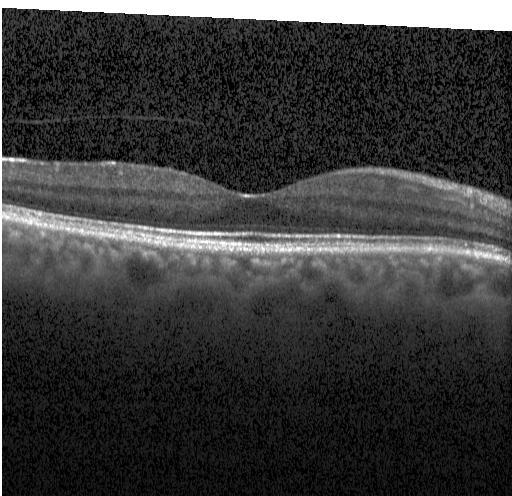

Retinal OCT B-scan
Finding: neither choroidal neovascularization, diabetic macular edema, nor drusen.